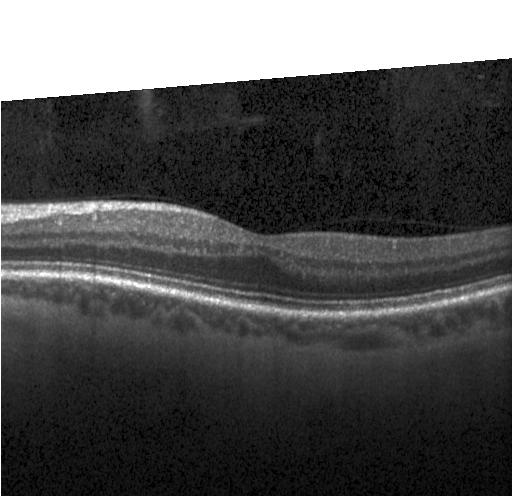 SD-OCT · optical coherence tomography scan · centered on the fovea — Diagnosis: no CNV, DME, or drusen.